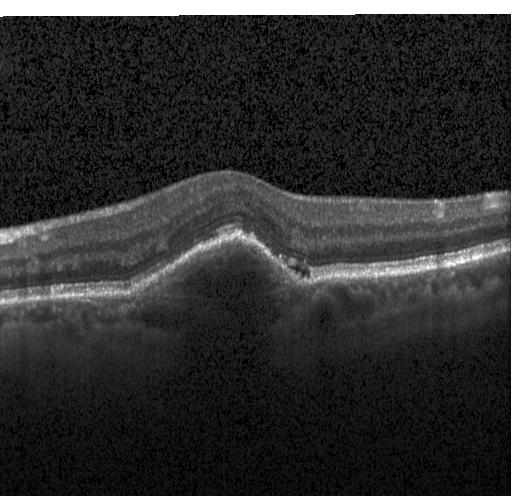 Instrument: Heidelberg Spectralis · spectral-domain OCT · fovea-centered · optical coherence tomography scan.
This B-scan demonstrates CNV.